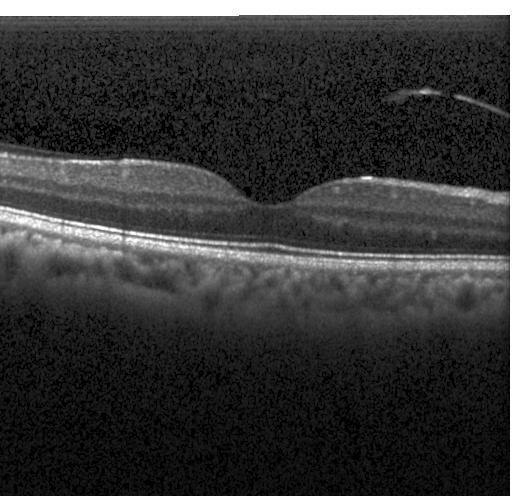 Macular OCT demonstrating no choroidal neovascularization, diabetic macular edema, or drusen.